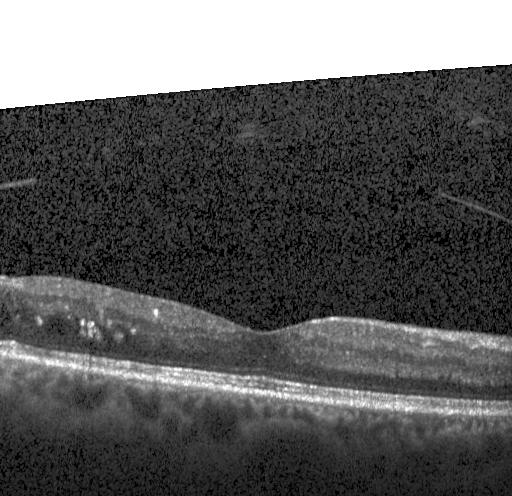
Macular OCT demonstrating diabetic macular edema (DME).